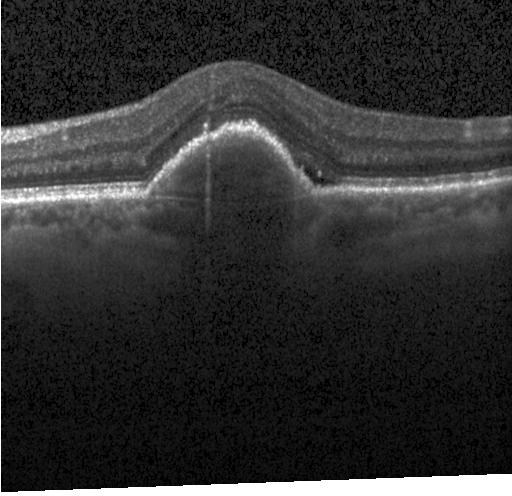

Spectral-domain OCT B-scan: choroidal neovascularization.